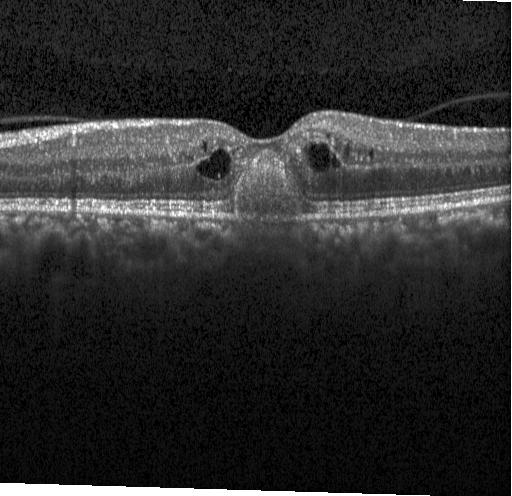
Spectral-domain optical coherence tomography, optical coherence tomography B-scan.
Diagnosis: a choroidal neovascular membrane.